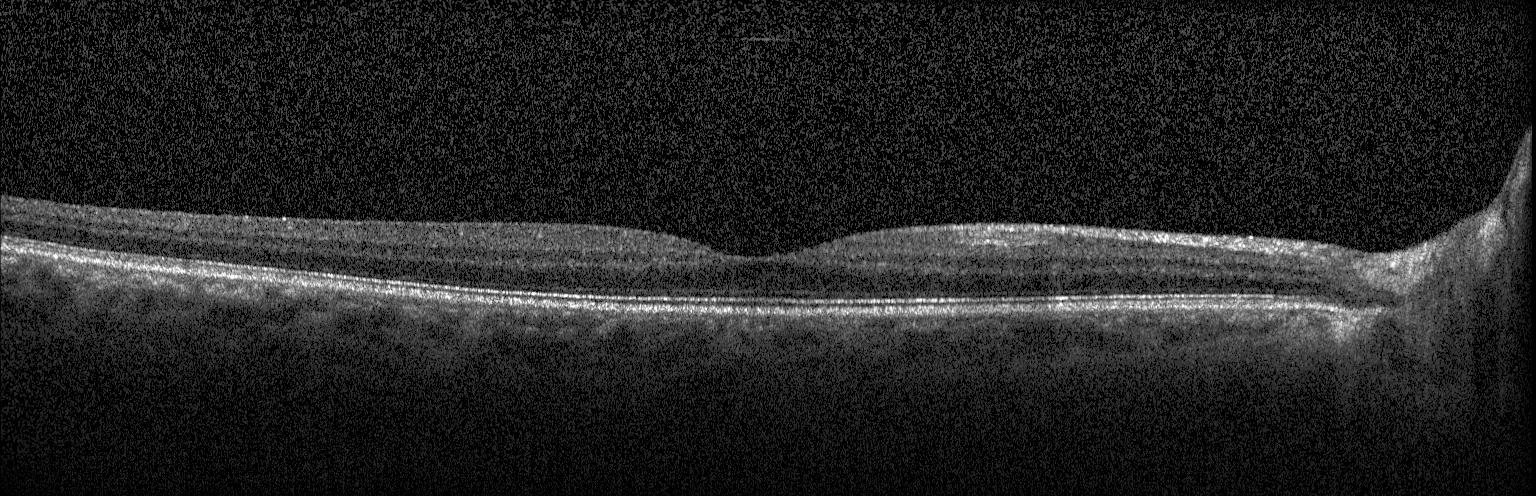

No CNV, no DME, and no drusen.